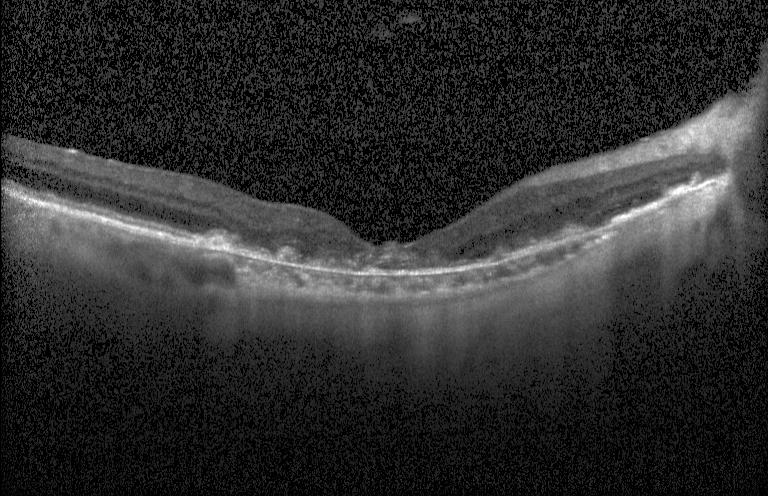

OCT line scan — Impression: CNV.